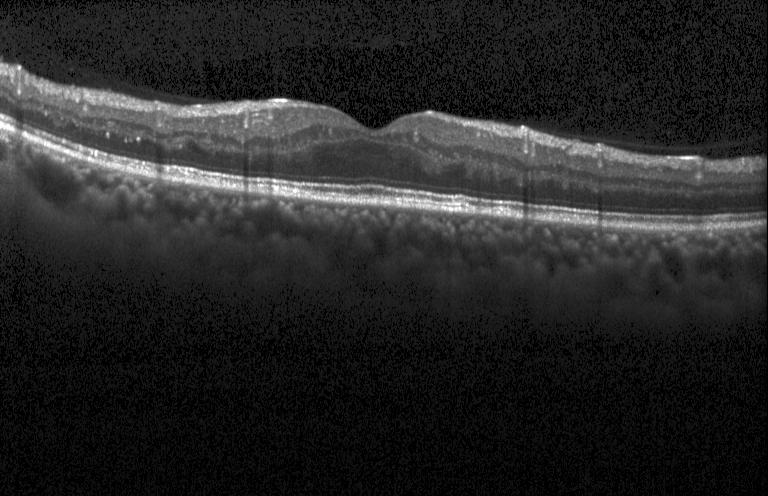

Optical coherence tomography scan
Finding: no evidence of choroidal neovascularization, diabetic macular edema, or drusen.